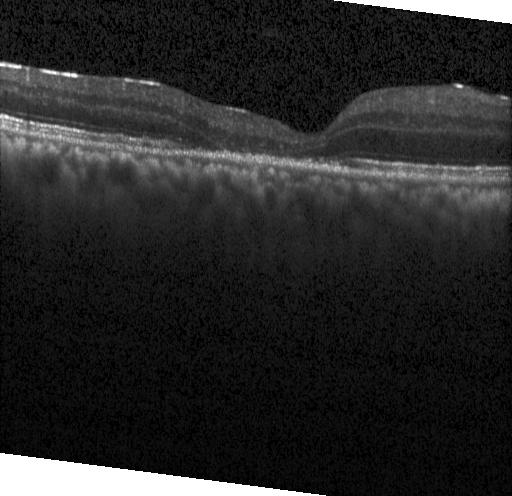

OCT line scan.
Diagnosis: neither CNV, DME, nor drusen.